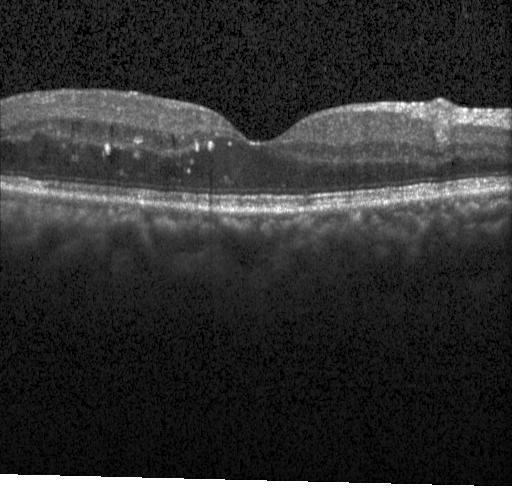

Retinal OCT cross-section. Horizontal scan through the fovea. SD-OCT. Diabetic macular edema (DME).